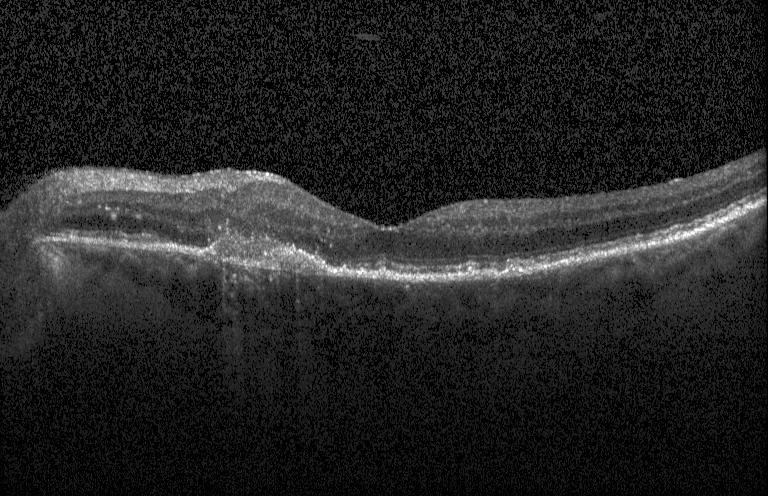 Centered on the fovea, OCT line scan.
Finding: a choroidal neovascular membrane.